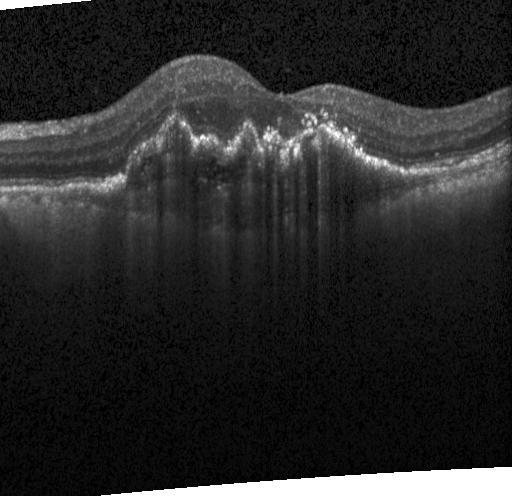

Dx: a choroidal neovascular membrane.